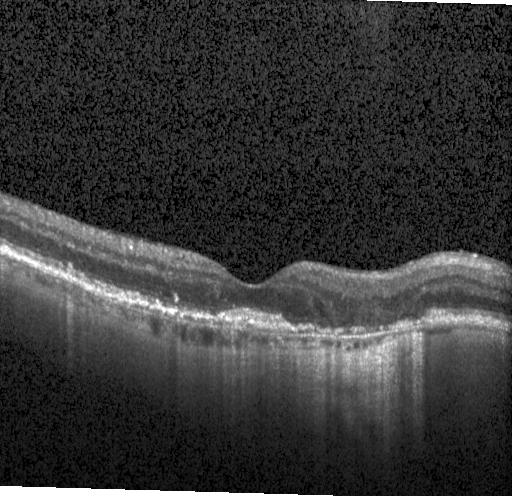

Retinal OCT B-scan, macular scan, spectral-domain optical coherence tomography, instrument: Heidelberg Spectralis
Macular OCT: choroidal neovascularization.